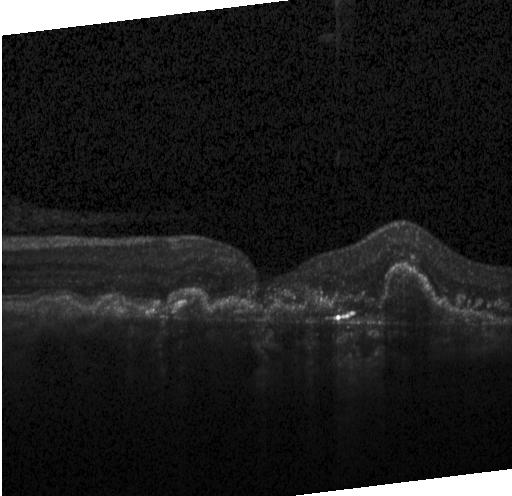
Heidelberg Spectralis OCT system; SD-OCT; retinal OCT B-scan; macular scan — Impression: a choroidal neovascular membrane.